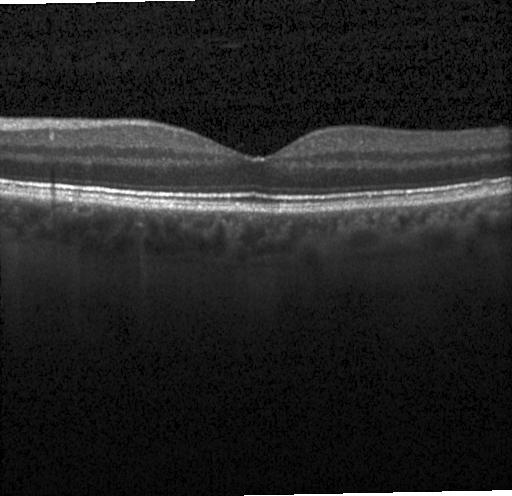 Retinal OCT B-scan. Horizontal scan through the fovea. Impression: no CNV, DME, or drusen.